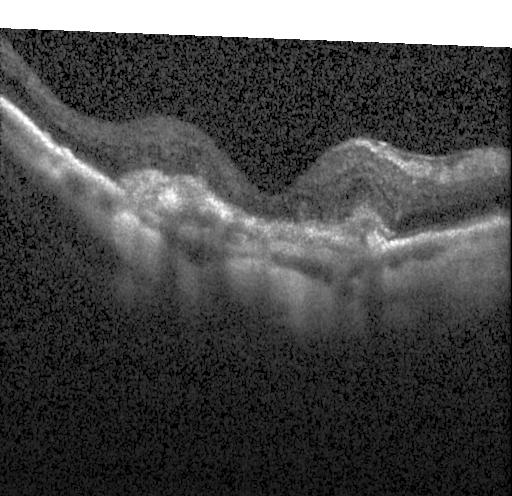 OCT line scan
Impression: CNV.